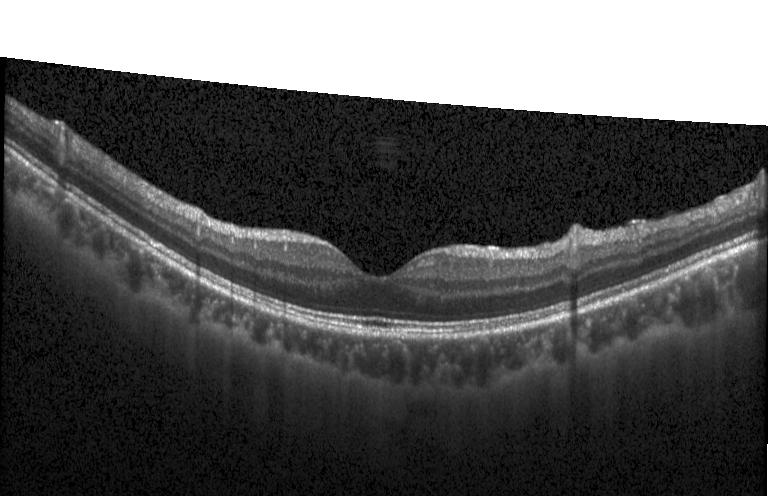

OCT scan showing no choroidal neovascularization, no diabetic macular edema, and no drusen.